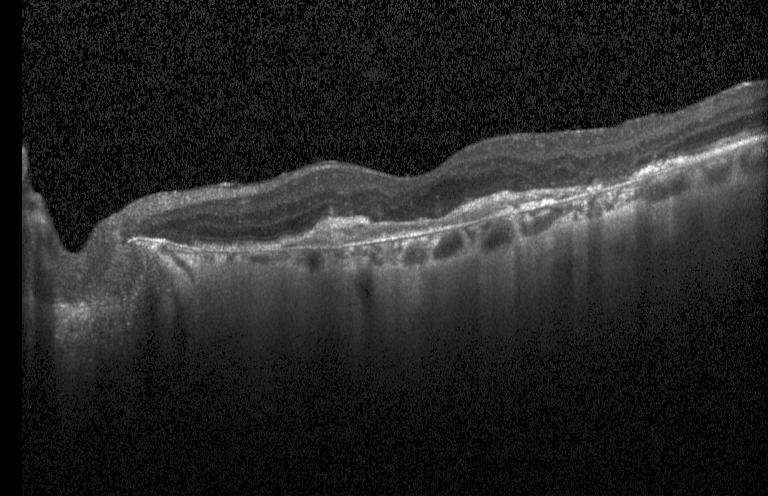
Heidelberg Spectralis OCT system; retinal OCT B-scan; SD-OCT; fovea-centered
Macular OCT: CNV.